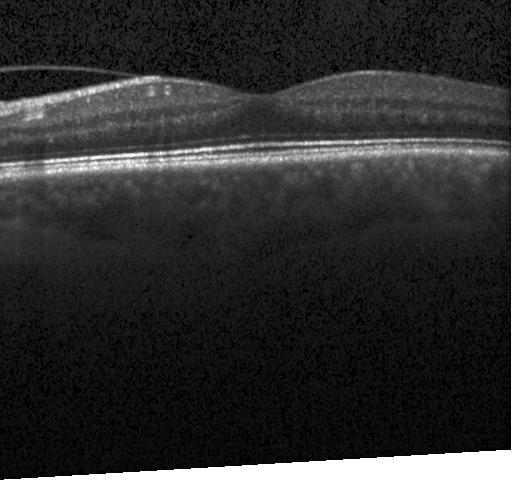 This B-scan demonstrates no evidence of choroidal neovascularization, diabetic macular edema, or drusen.